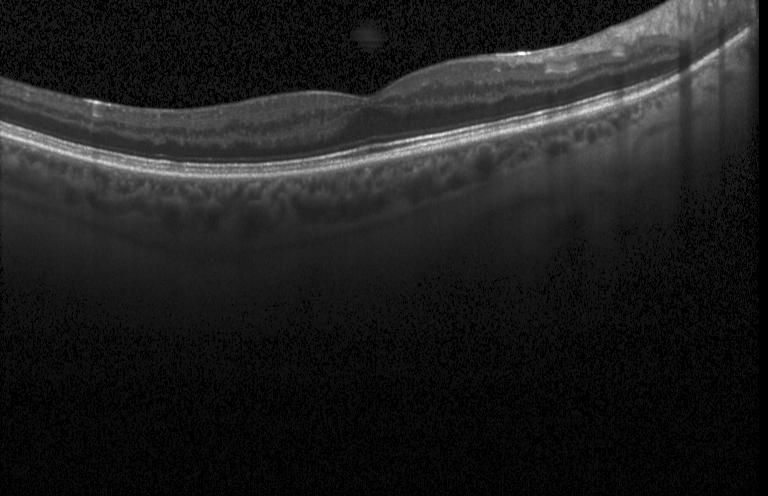 The scan shows no CNV, DME, or drusen.